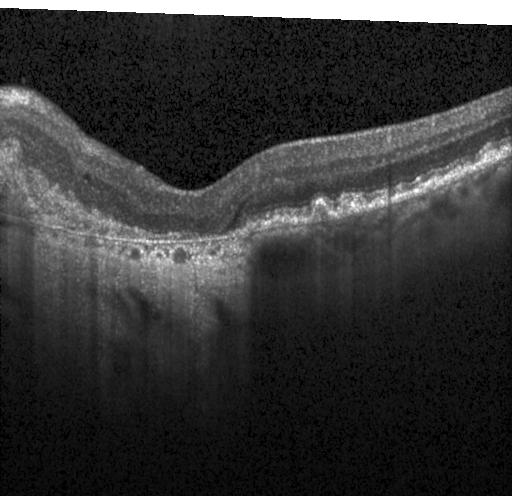

Spectral-domain OCT B-scan: choroidal neovascularization.